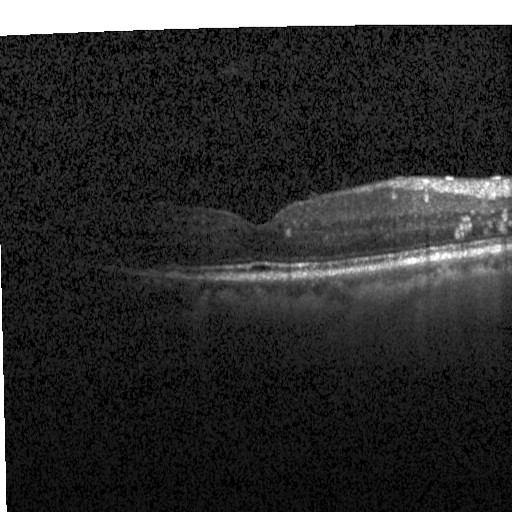 Diagnosis: diabetic macular edema.